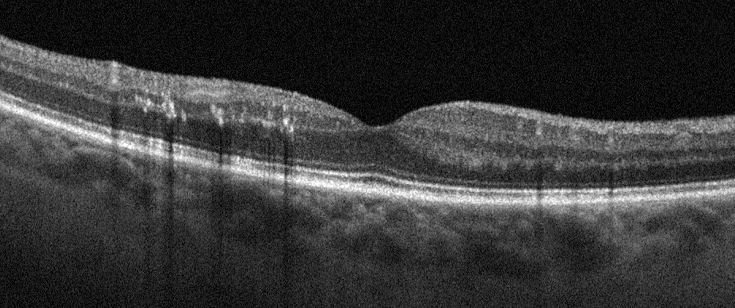

Optical coherence tomography scan, through the macula.
Diabetic macular edema.